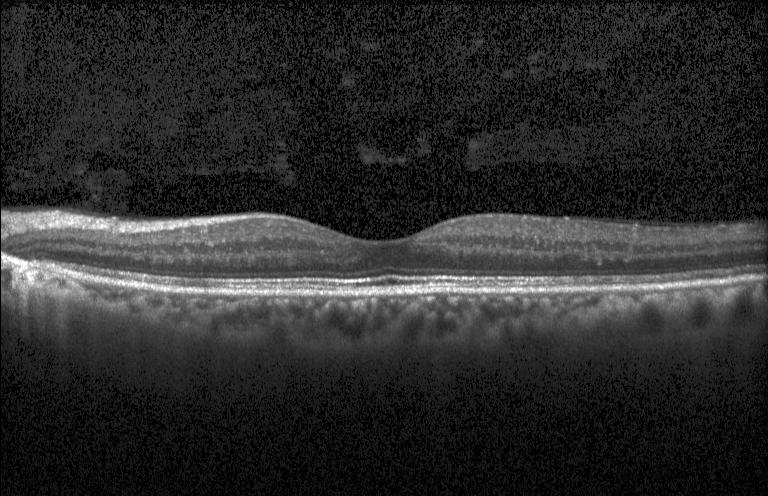 Retinal OCT cross-section. The scan shows no CNV, DME, or drusen.